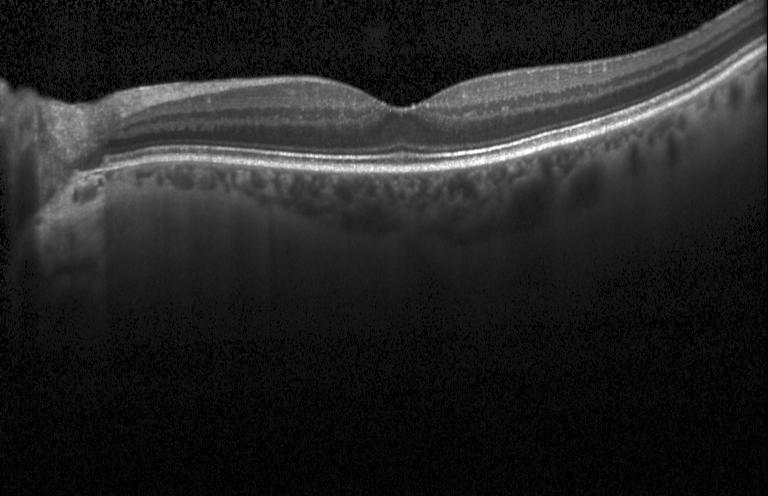
Heidelberg Spectralis OCT system; retinal OCT cross-section
Impression: neither CNV, DME, nor drusen.